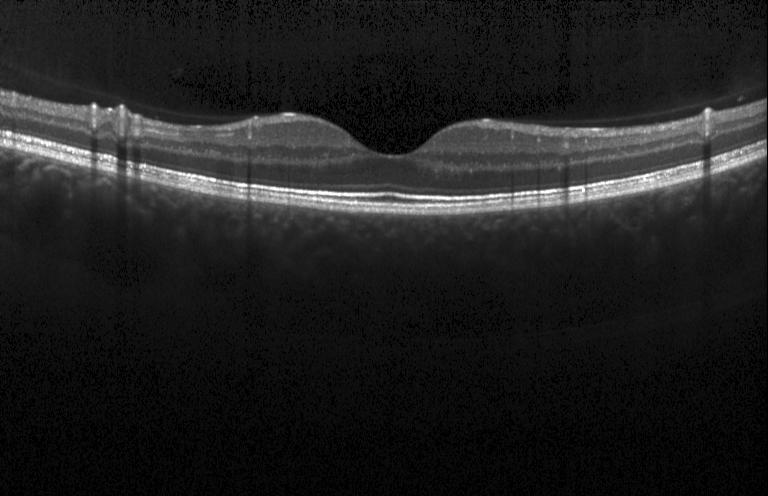
Neither choroidal neovascularization, diabetic macular edema, nor drusen.